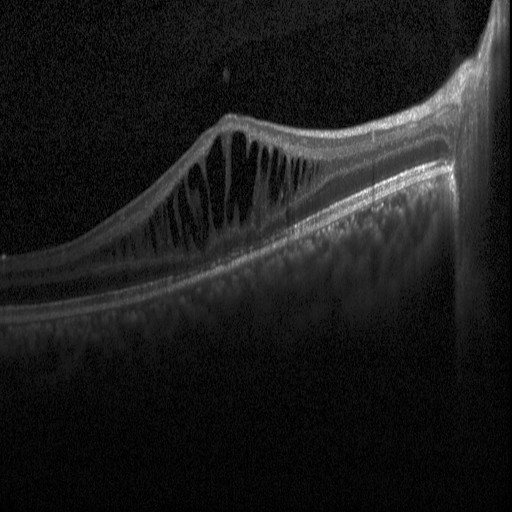
OCT B-scan. Horizontal scan through the fovea
Finding: diabetic macular edema (DME).